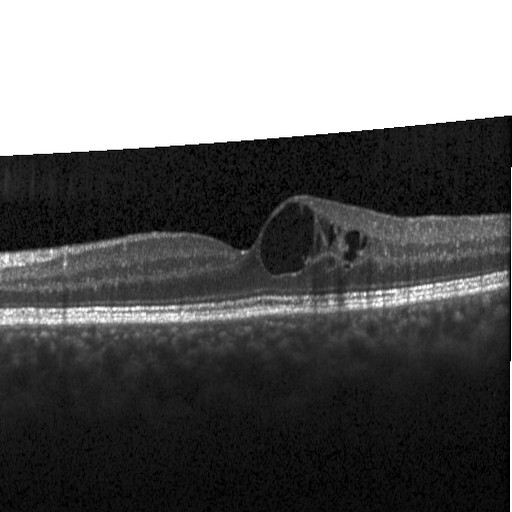

OCT line scan · through the macula · Heidelberg Spectralis · spectral-domain optical coherence tomography.
Macular OCT: DME.